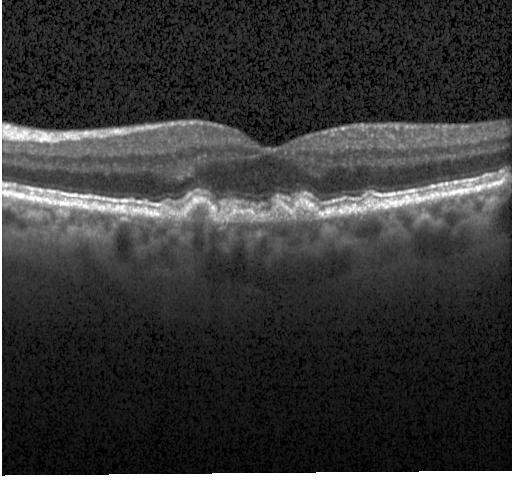 OCT B-scan
Diagnosis: drusen.